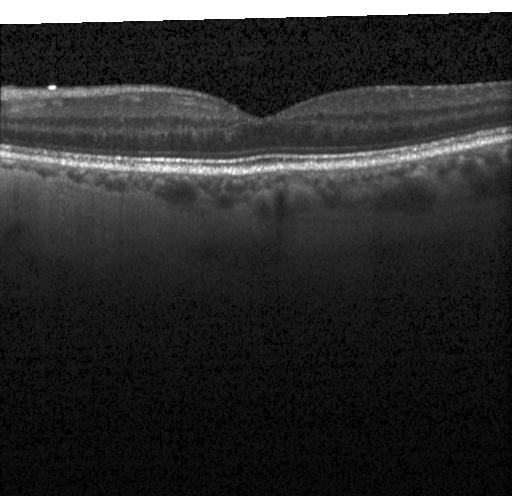 Through the macula, retinal OCT cross-section. Impression: no choroidal neovascularization, diabetic macular edema, or drusen.